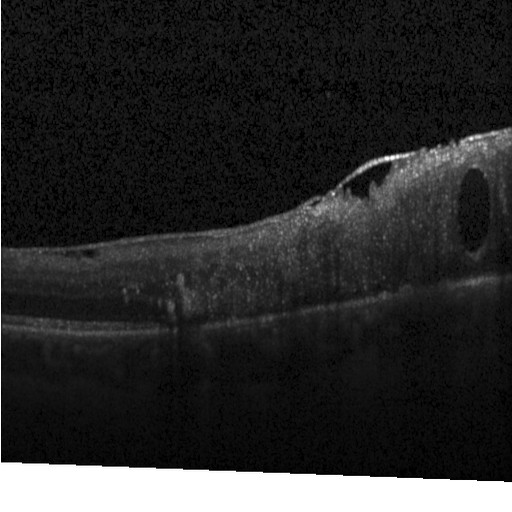

Optical coherence tomography B-scan, centered on the fovea. OCT finding: diabetic macular edema.